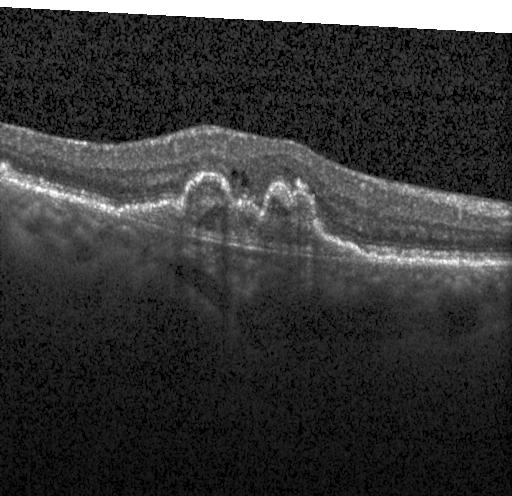

Spectral-domain OCT · instrument: Heidelberg Spectralis · fovea-centered · optical coherence tomography scan. A choroidal neovascular membrane.